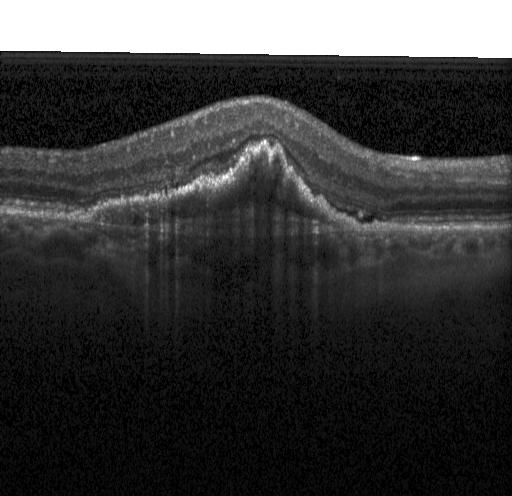 Retinal OCT B-scan; SD-OCT; fovea-centered; instrument: Heidelberg Spectralis. Impression: choroidal neovascularization (CNV).